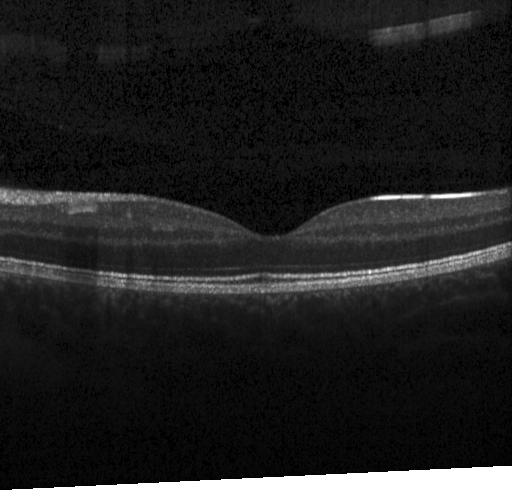

OCT B-scan · macular scan — Impression: no CNV, no DME, and no drusen.